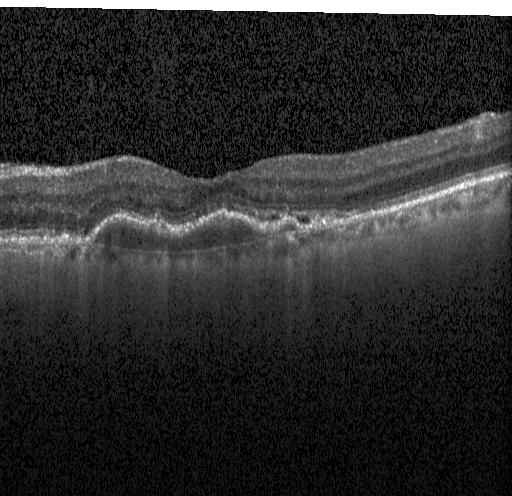
OCT scan showing a choroidal neovascular membrane.